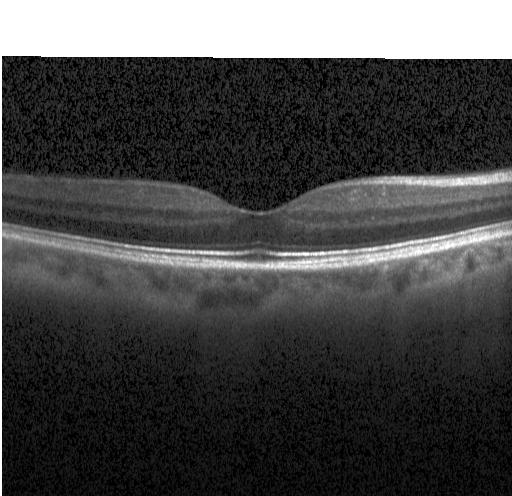
Retinal OCT cross-section
Finding: neither choroidal neovascularization, diabetic macular edema, nor drusen.